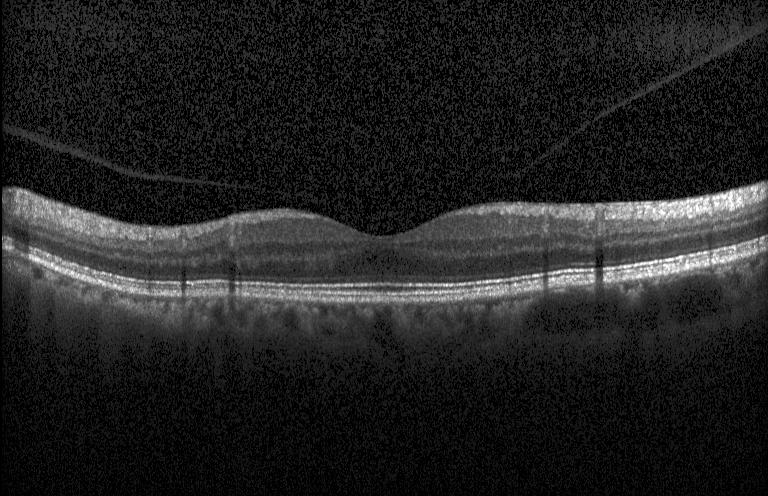
Heidelberg Spectralis OCT system. SD-OCT. Retinal OCT cross-section. Diagnosis: no choroidal neovascularization, no diabetic macular edema, and no drusen.